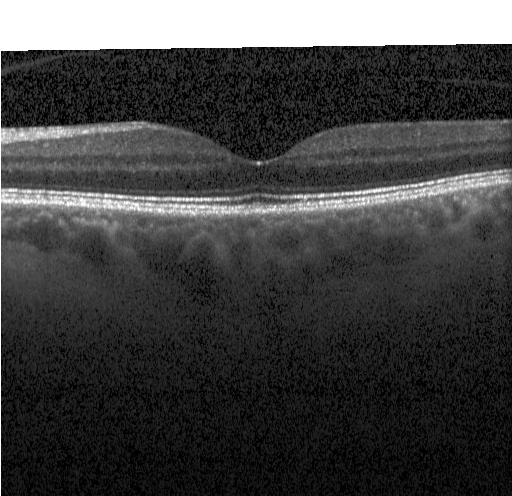 Finding: no evidence of choroidal neovascularization, diabetic macular edema, or drusen.